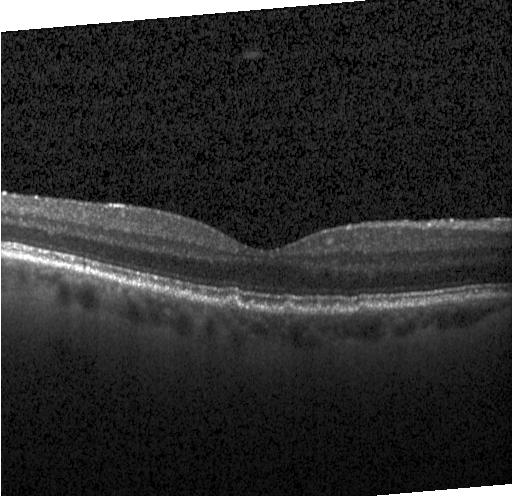
Instrument: Heidelberg Spectralis, centered on the fovea, spectral-domain OCT, optical coherence tomography scan — The scan shows drusen.